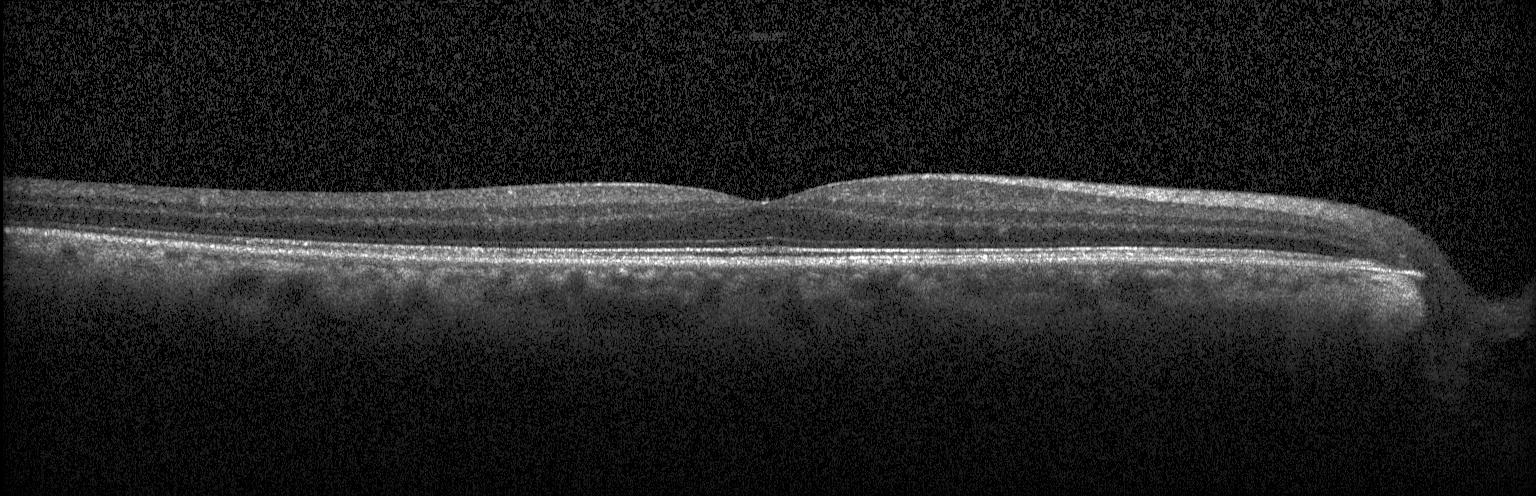

OCT B-scan — Finding: no choroidal neovascularization, diabetic macular edema, or drusen.